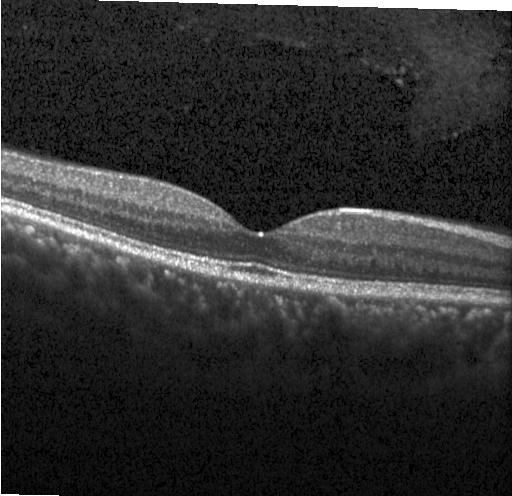 OCT line scan. Spectral-domain OCT
Finding: neither choroidal neovascularization, diabetic macular edema, nor drusen.